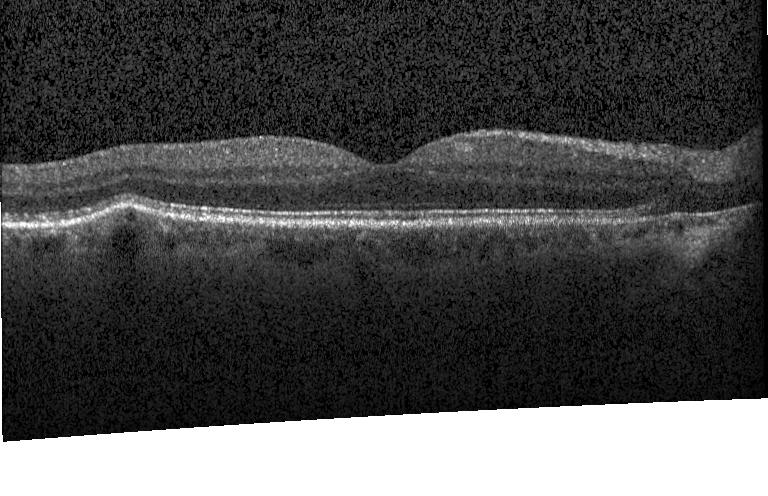

OCT line scan; fovea-centered; spectral-domain OCT; Heidelberg Spectralis OCT system. Assessment: no evidence of choroidal neovascularization, diabetic macular edema, or drusen.